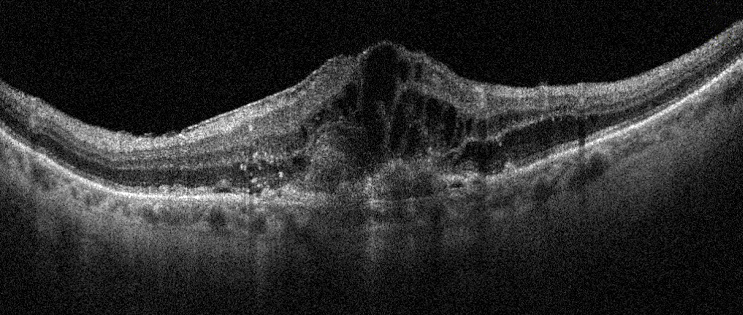

Optical coherence tomography B-scan · fovea-centered — AMD.